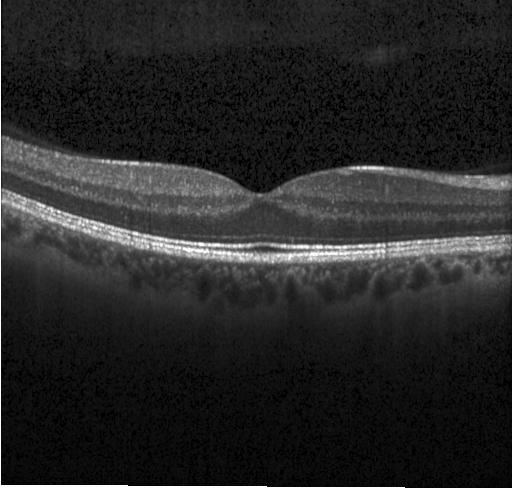 Retinal OCT B-scan; instrument: Heidelberg Spectralis; SD-OCT; macular scan.
Assessment: no choroidal neovascularization, diabetic macular edema, or drusen.